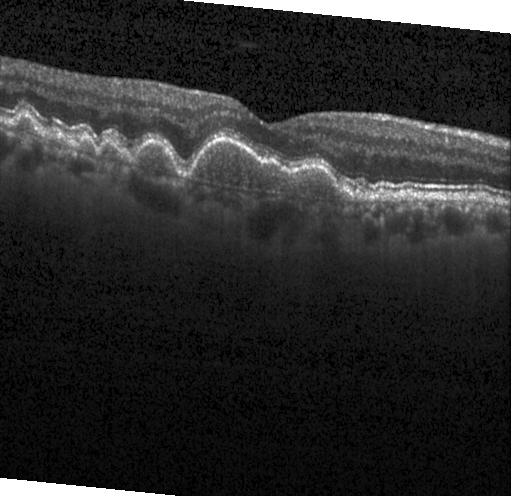 OCT line scan; spectral-domain OCT; Heidelberg Spectralis OCT system.
Diagnosis: sub-RPE drusenoid deposits.